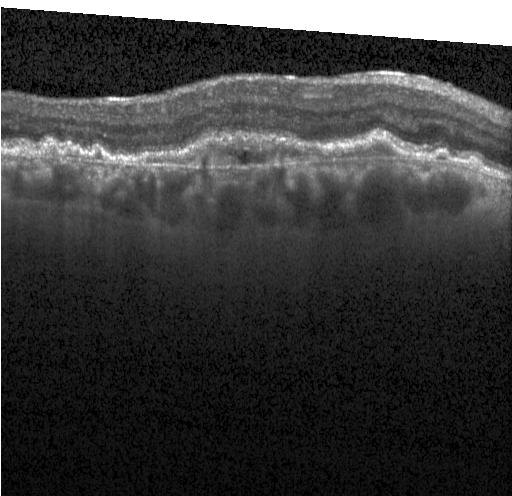

Retinal OCT B-scan. The scan shows choroidal neovascularization.